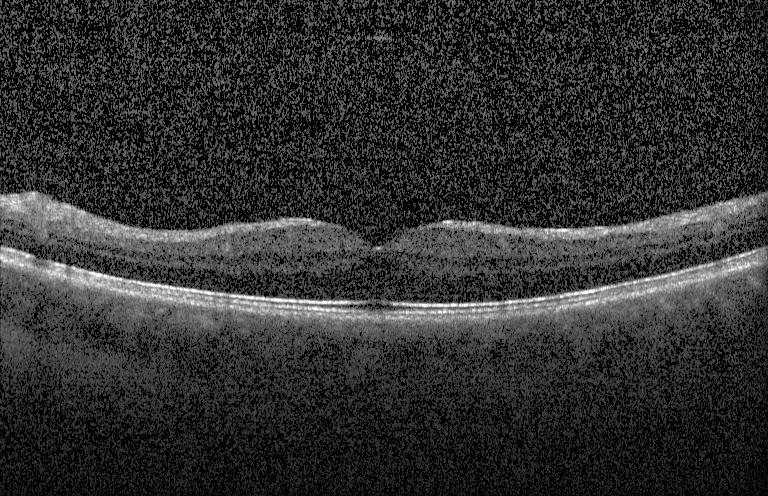
Heidelberg Spectralis; through the macula; retinal OCT B-scan; SD-OCT
Finding: no choroidal neovascularization, diabetic macular edema, or drusen.